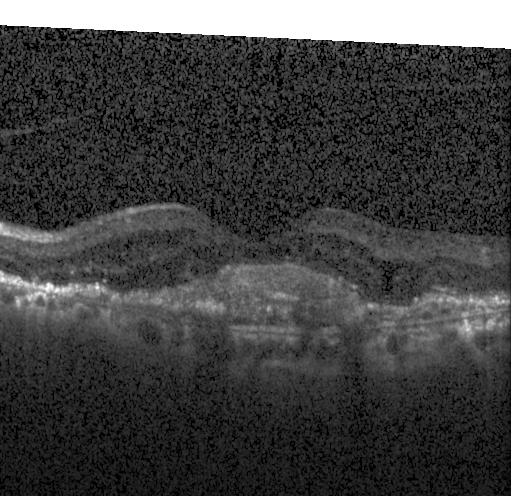 Heidelberg Spectralis · SD-OCT · OCT B-scan · horizontal scan through the fovea.
Impression: choroidal neovascularization.